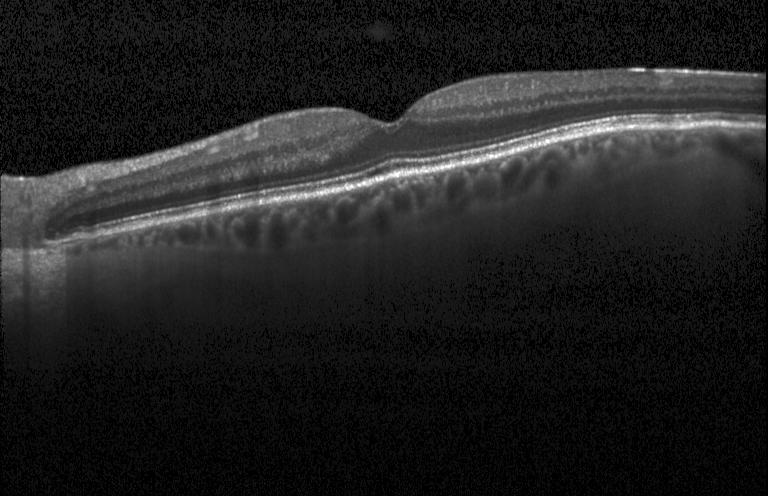 Retinal OCT cross-section.
Finding: no choroidal neovascularization, diabetic macular edema, or drusen.